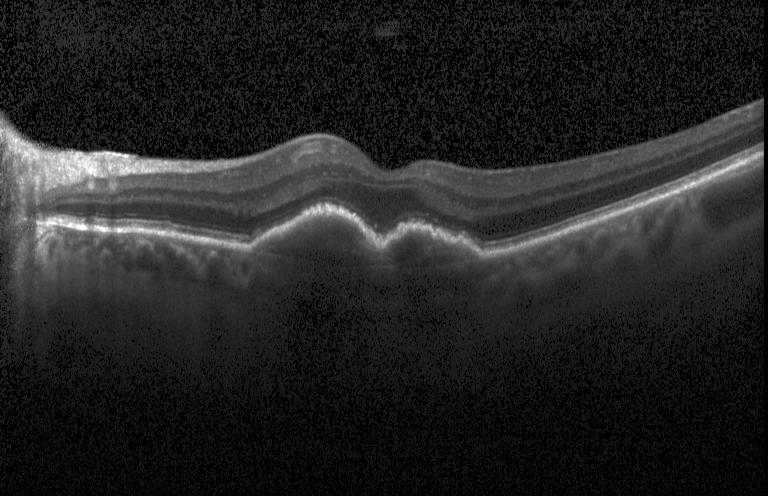 Assessment: CNV.